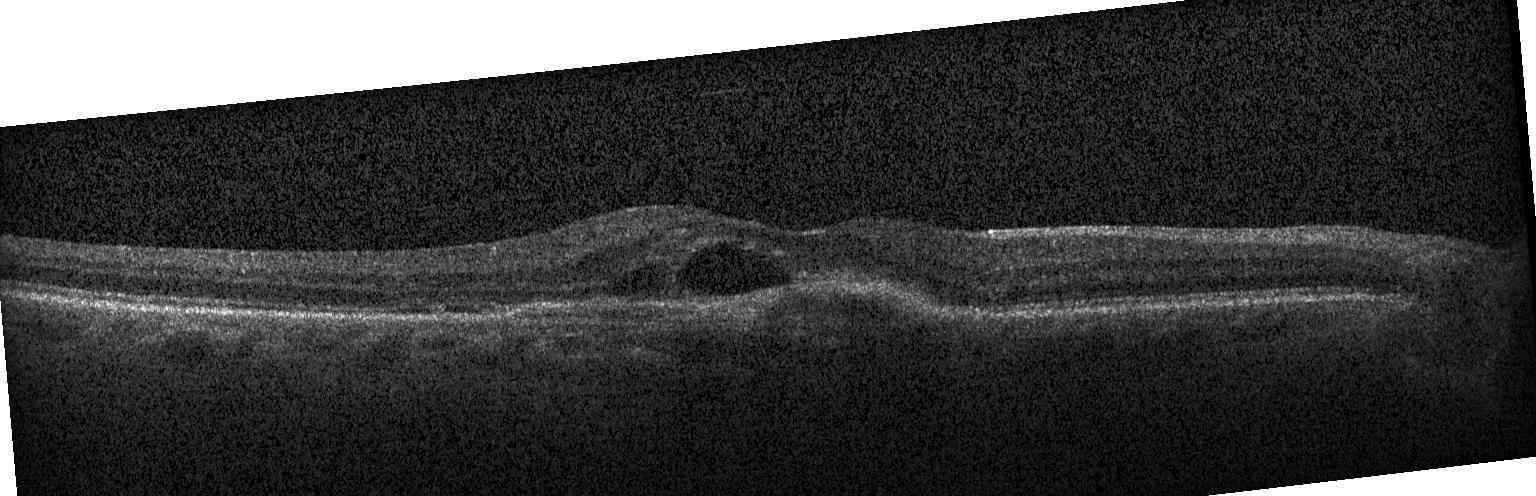 A choroidal neovascular membrane.